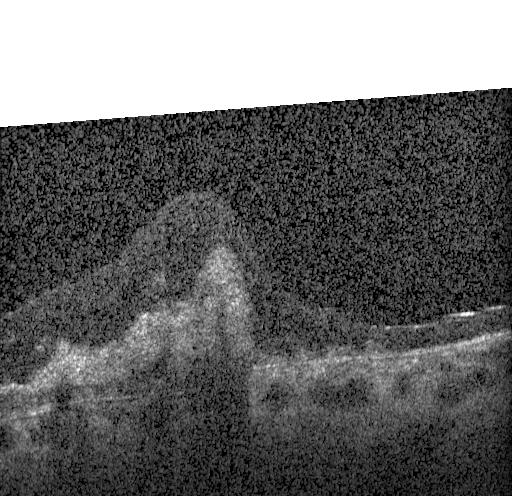

OCT B-scan, spectral-domain optical coherence tomography, horizontal scan through the fovea, acquired on a Heidelberg Spectralis — The scan shows a choroidal neovascular membrane.